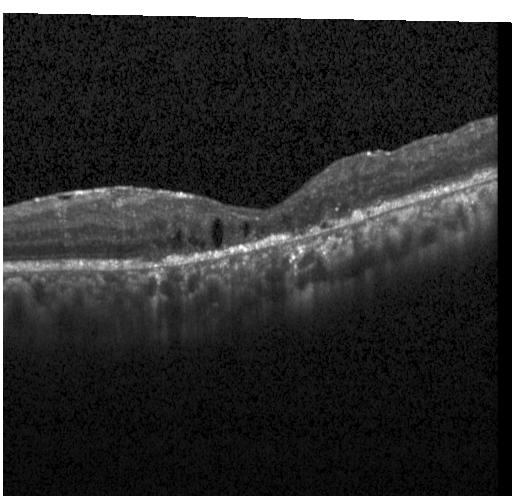
A choroidal neovascular membrane.